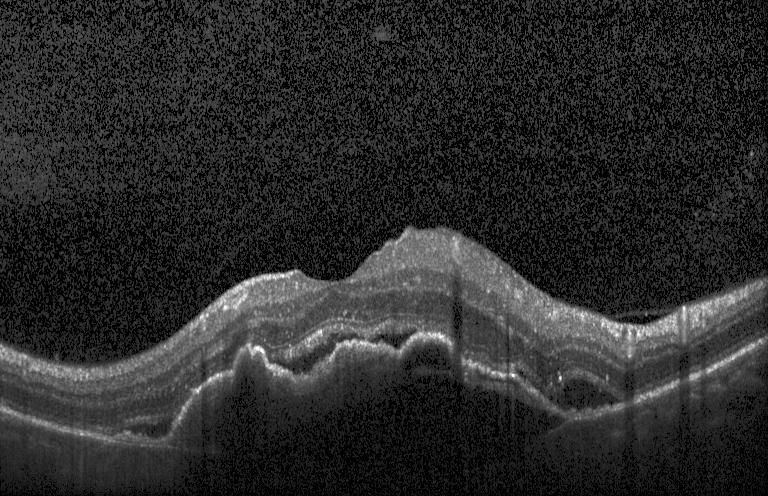

Heidelberg Spectralis OCT system · retinal OCT cross-section · horizontal scan through the fovea · spectral-domain optical coherence tomography.
Finding: CNV.